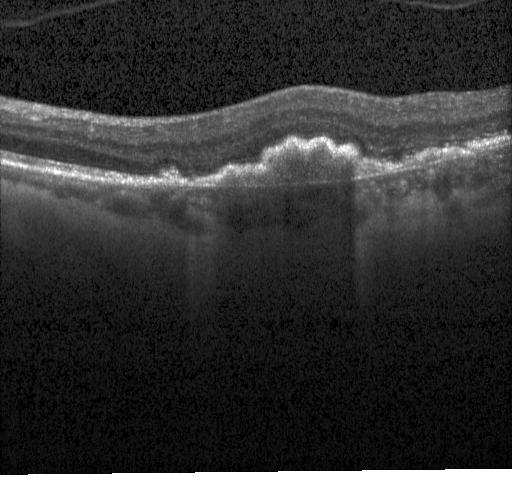 Finding: a choroidal neovascular membrane.